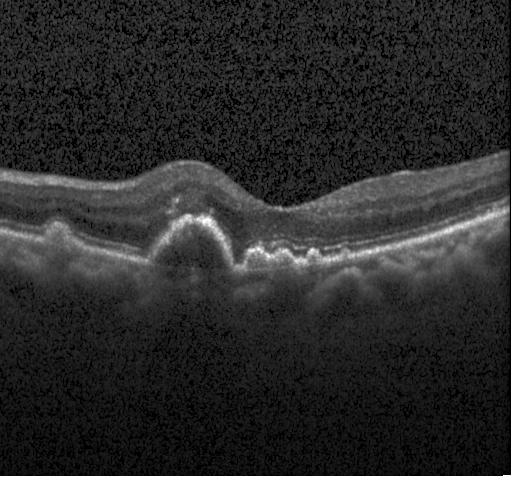

Retinal OCT B-scan.
This B-scan demonstrates drusen.